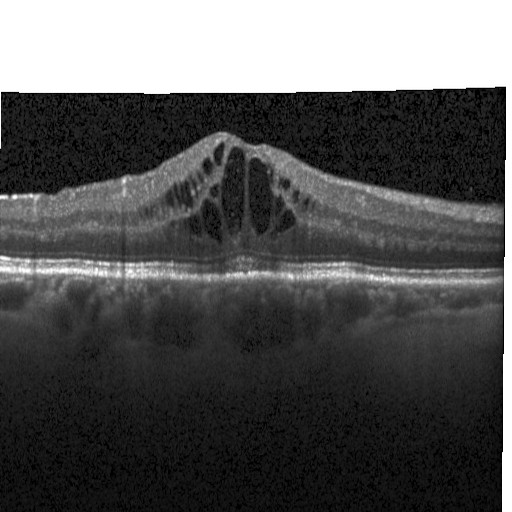

OCT scan showing diabetic macular edema (DME).